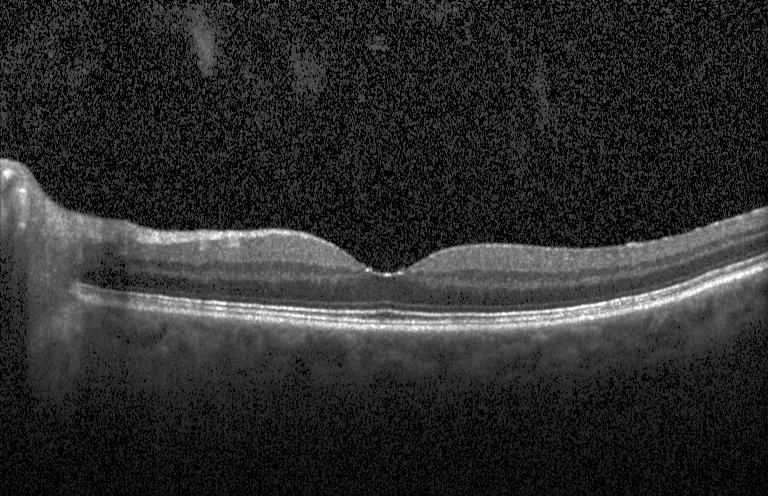
Optical coherence tomography B-scan
Dx: no evidence of choroidal neovascularization, diabetic macular edema, or drusen.